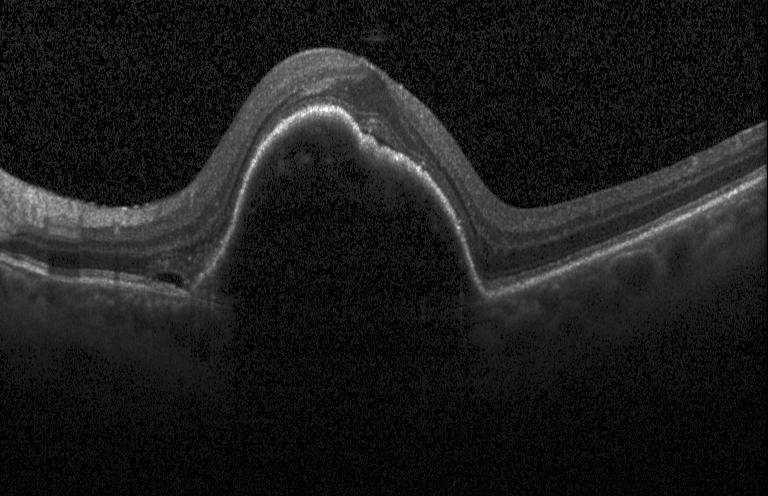
Spectral-domain optical coherence tomography, macular scan, acquired on a Heidelberg Spectralis, optical coherence tomography scan. Finding: choroidal neovascularization (CNV).